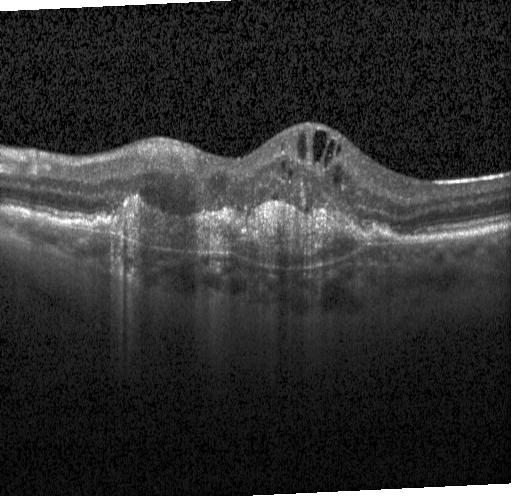
Centered on the fovea · Heidelberg Spectralis OCT system · retinal OCT B-scan — OCT finding: a choroidal neovascular membrane.